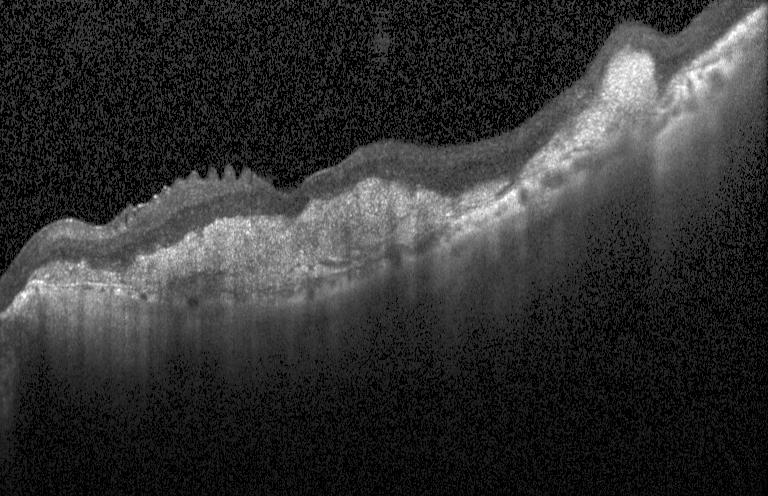
Fovea-centered, spectral-domain OCT, retinal OCT cross-section
Impression: CNV.